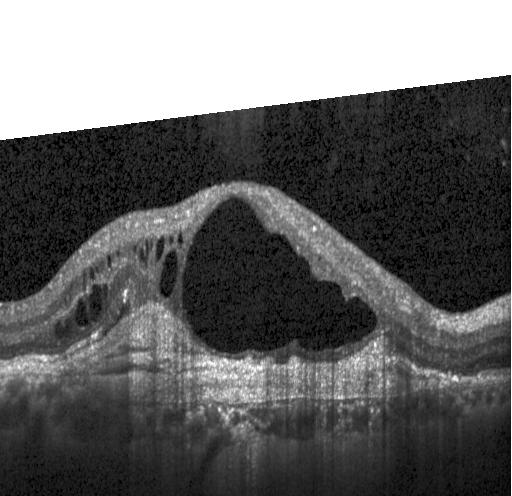
Finding: CNV.